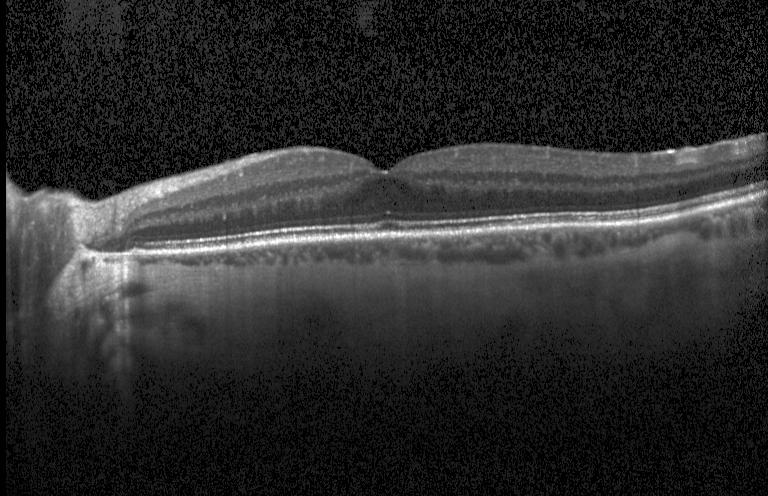 Optical coherence tomography B-scan, macular scan, spectral-domain OCT — OCT finding: no CNV, no DME, and no drusen.